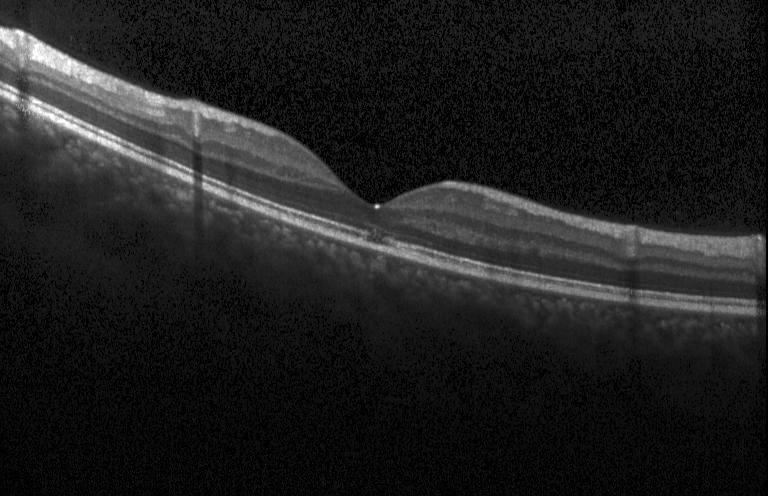 Diagnosis: no choroidal neovascularization, diabetic macular edema, or drusen.